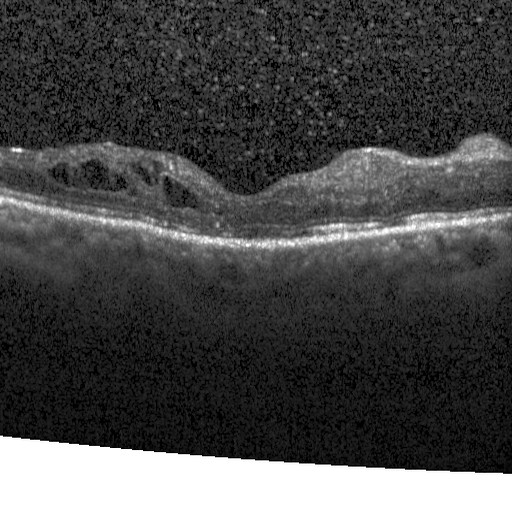
Diagnosis: diabetic macular edema (DME).